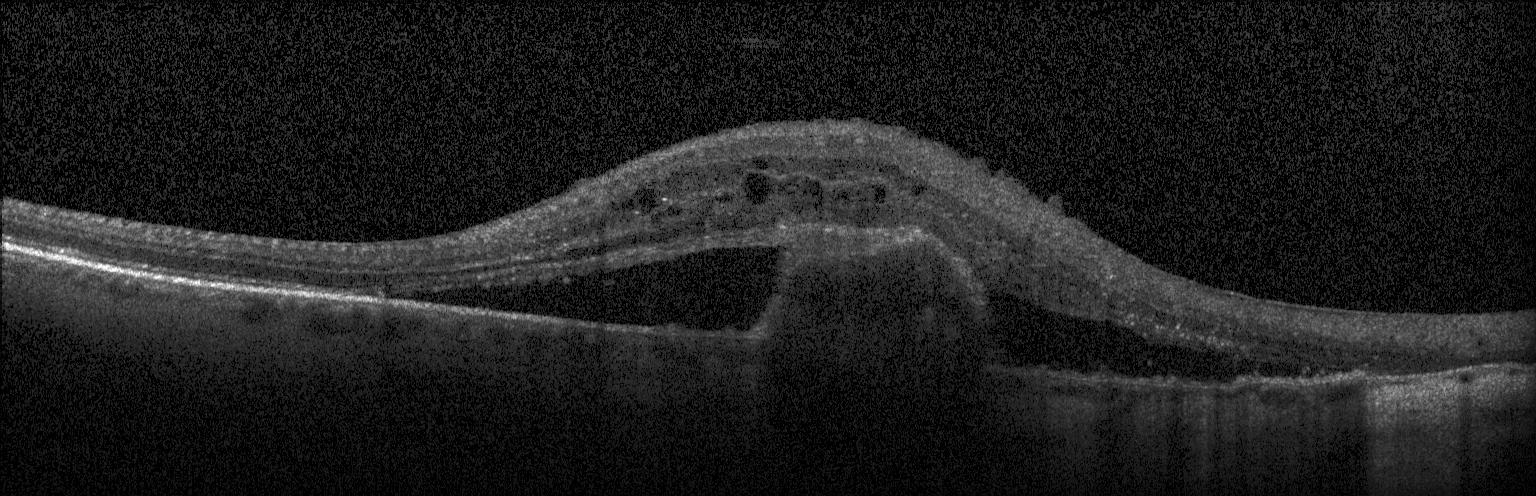
Optical coherence tomography scan; centered on the fovea.
This B-scan demonstrates choroidal neovascularization (CNV).